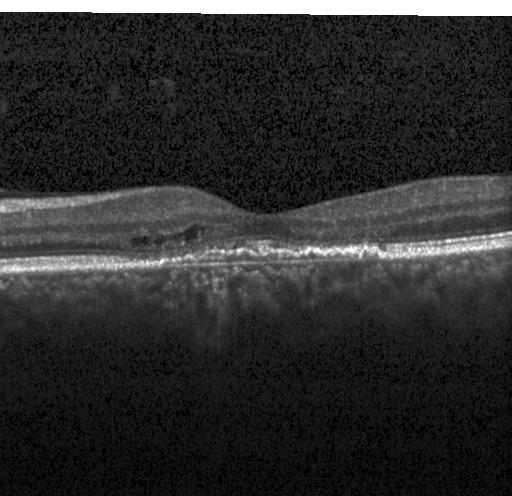
Impression: choroidal neovascularization.